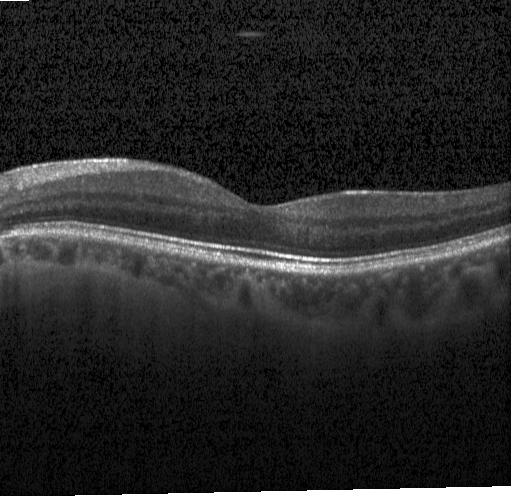

Spectral-domain OCT; fovea-centered; retinal OCT cross-section; instrument: Heidelberg Spectralis.
Diagnosis: no CNV, DME, or drusen.